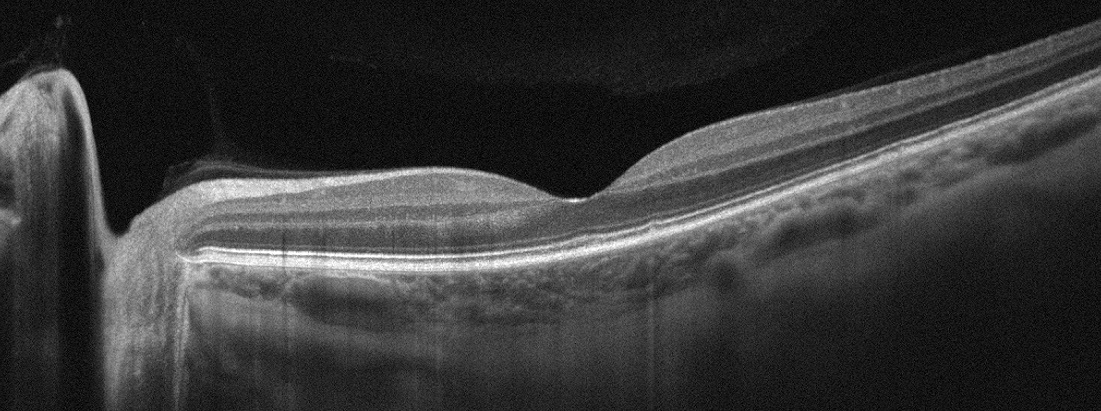
Retinal OCT cross-section.
Assessment: age-related macular degeneration (AMD).